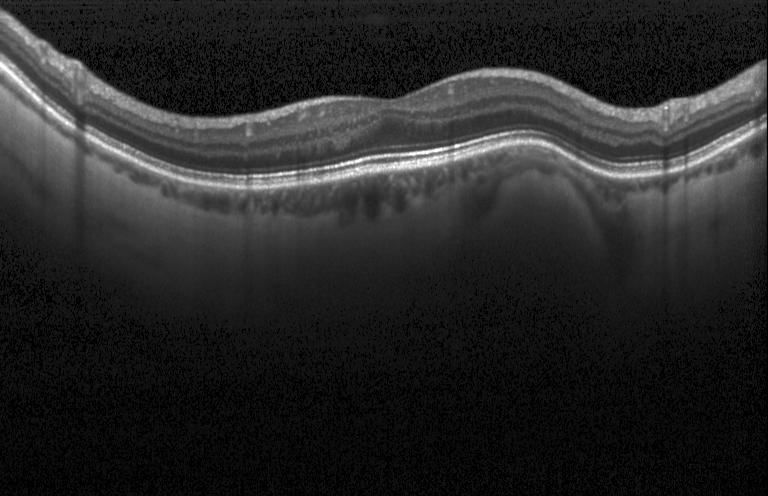

Macular OCT demonstrating no CNV, DME, or drusen.